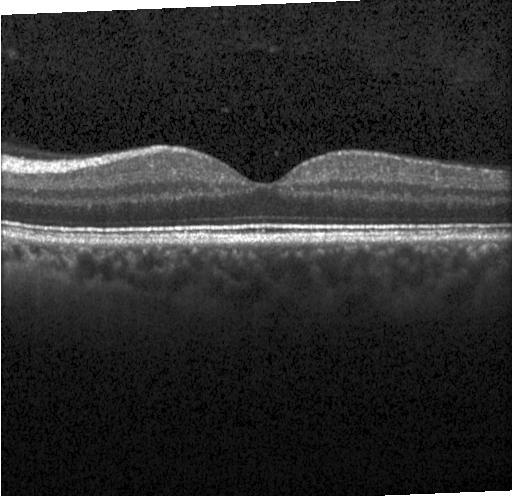

Optical coherence tomography B-scan.
Impression: no choroidal neovascularization, no diabetic macular edema, and no drusen.